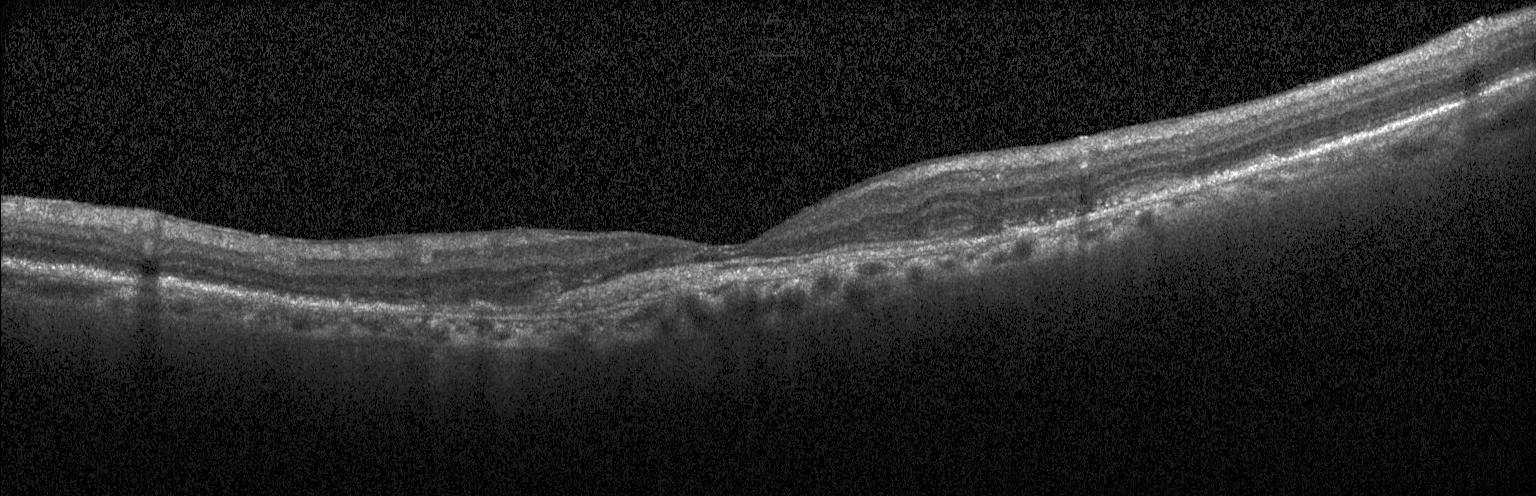

Optical coherence tomography B-scan; instrument: Heidelberg Spectralis — This B-scan demonstrates choroidal neovascularization (CNV).